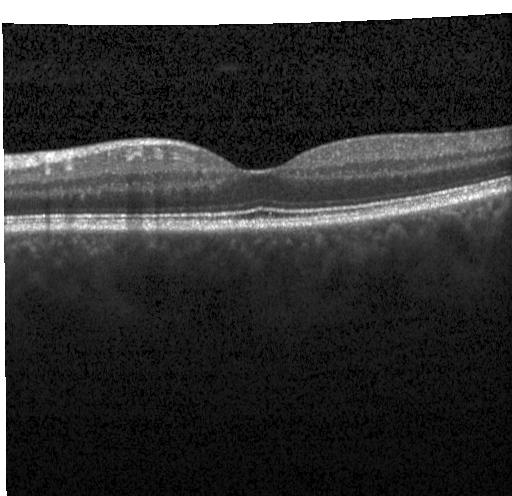
Impression: no choroidal neovascularization, no diabetic macular edema, and no drusen.